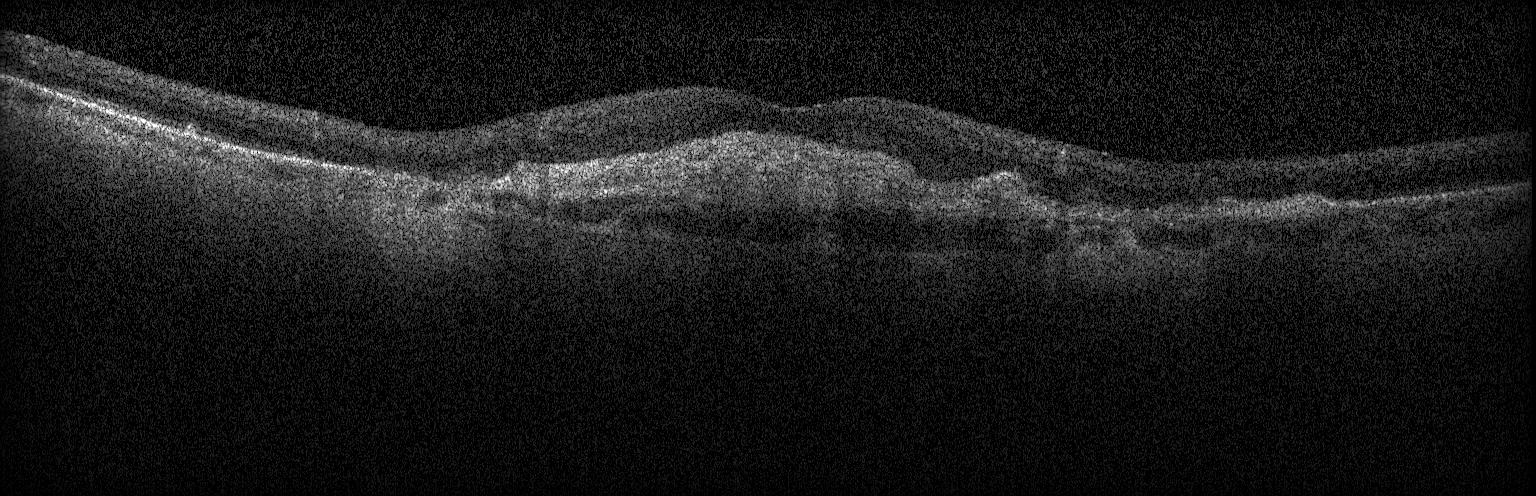 Dx: a choroidal neovascular membrane.